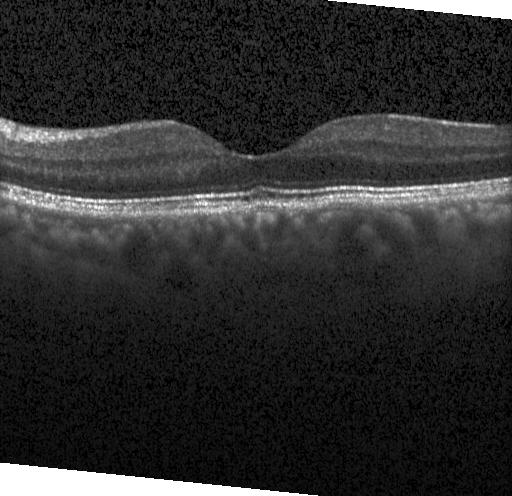 OCT line scan.
The scan shows neither CNV, DME, nor drusen.